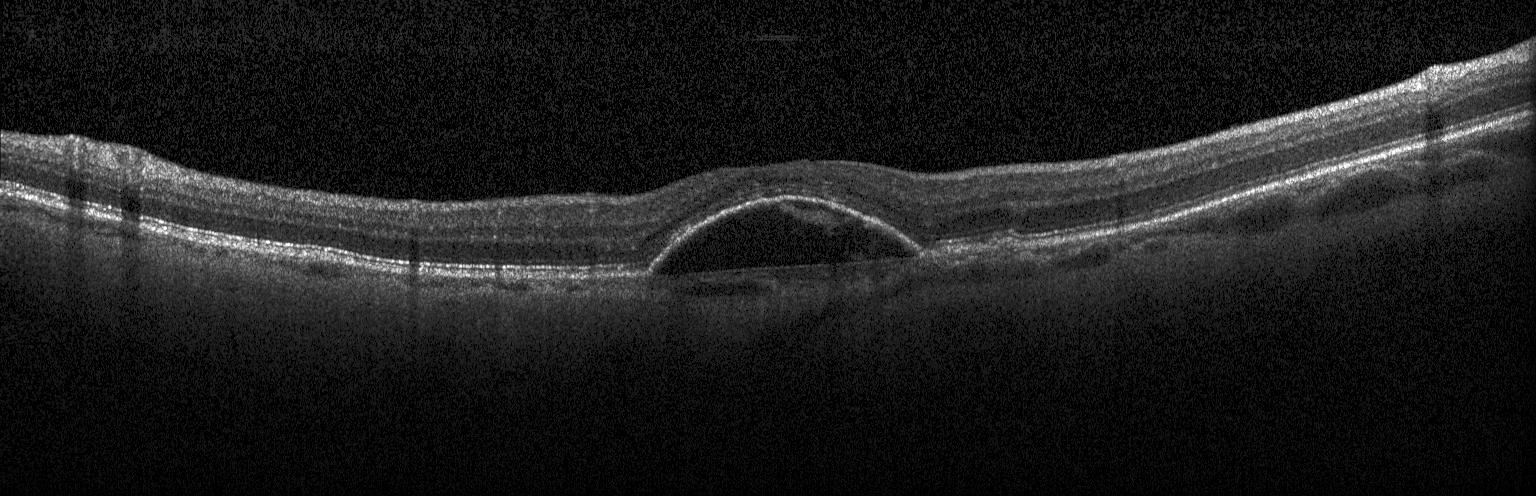

OCT B-scan, centered on the fovea, instrument: Heidelberg Spectralis. Impression: a choroidal neovascular membrane.